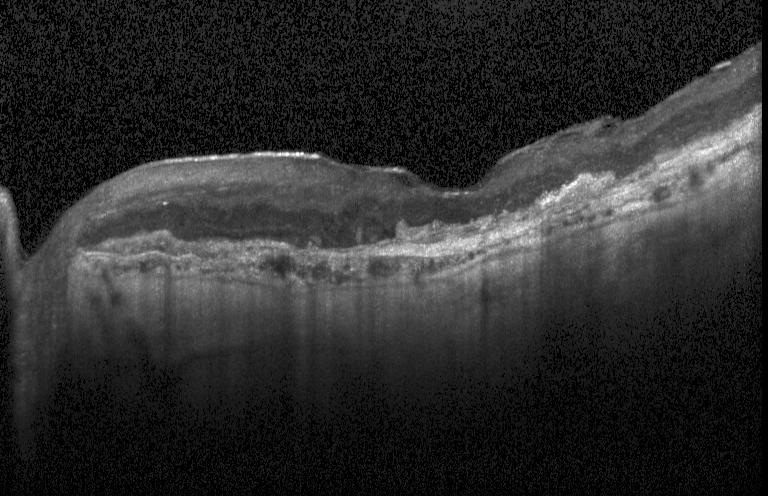 Optical coherence tomography B-scan
Diagnosis: a choroidal neovascular membrane.